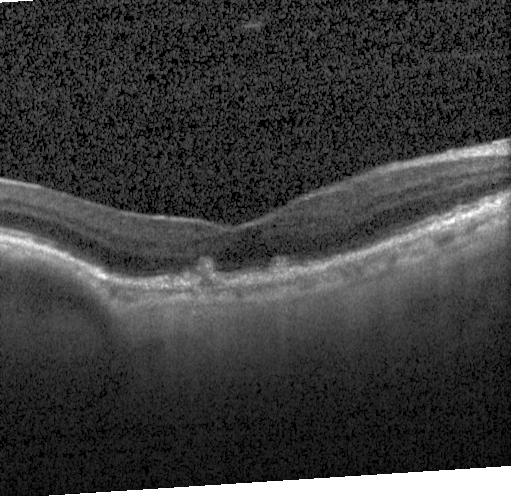
Centered on the fovea · spectral-domain optical coherence tomography · optical coherence tomography B-scan. Assessment: a choroidal neovascular membrane.